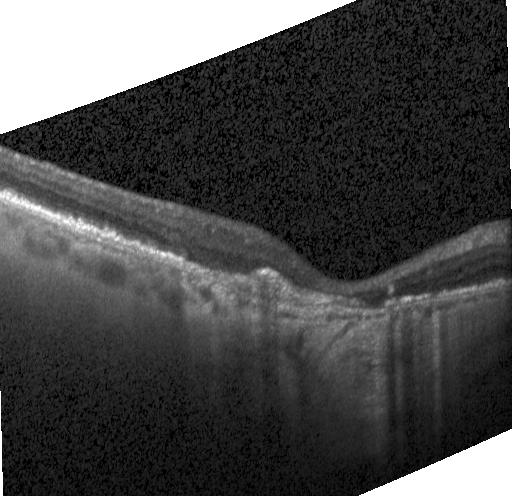 Optical coherence tomography scan
This B-scan demonstrates a choroidal neovascular membrane.